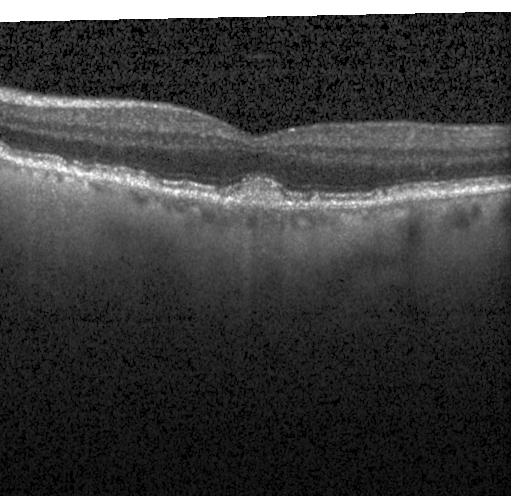 Impression: sub-RPE drusenoid deposits.